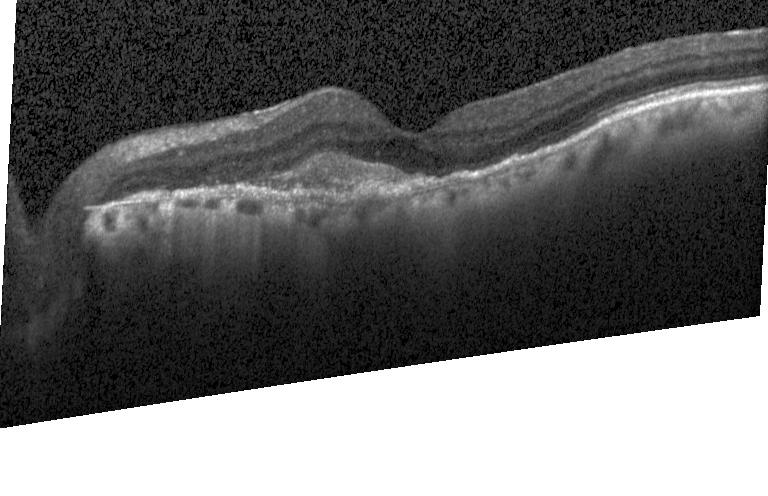

Diagnosis: choroidal neovascularization (CNV).